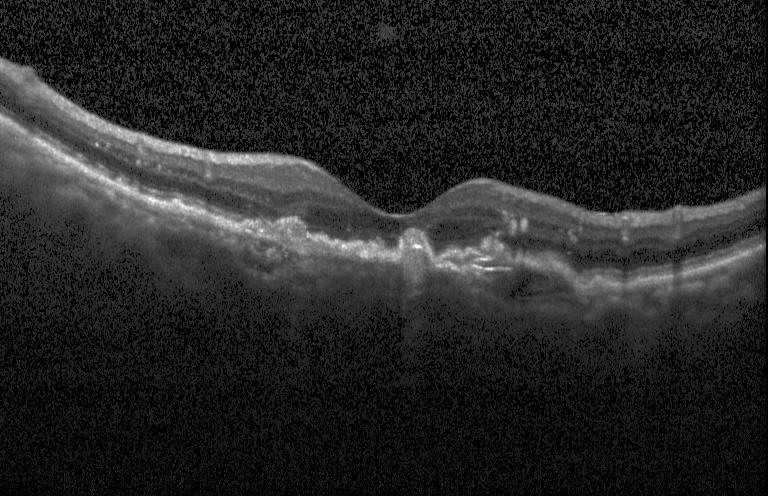
Retinal OCT cross-section showing choroidal neovascularization (CNV).